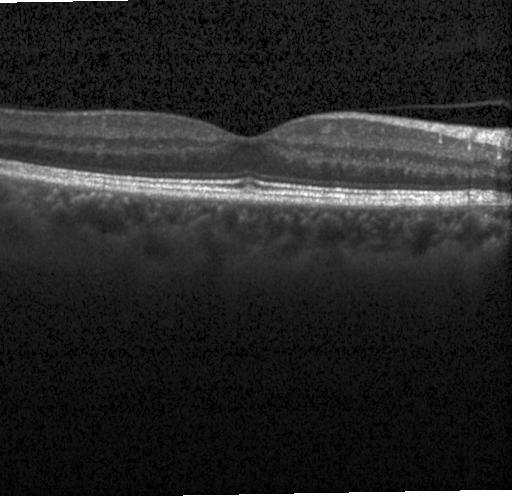

Spectral-domain OCT B-scan: no CNV, DME, or drusen.